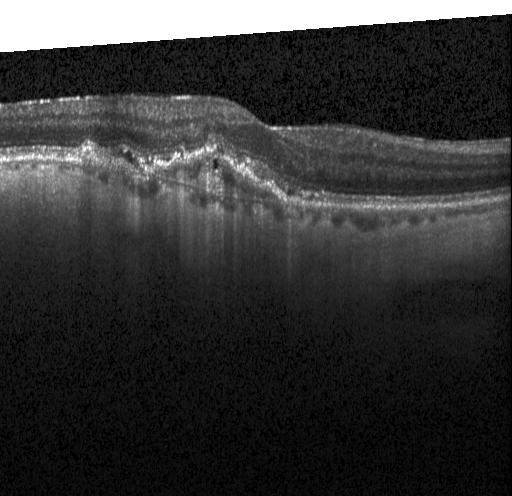

Heidelberg Spectralis OCT system · OCT line scan
Assessment: a choroidal neovascular membrane.